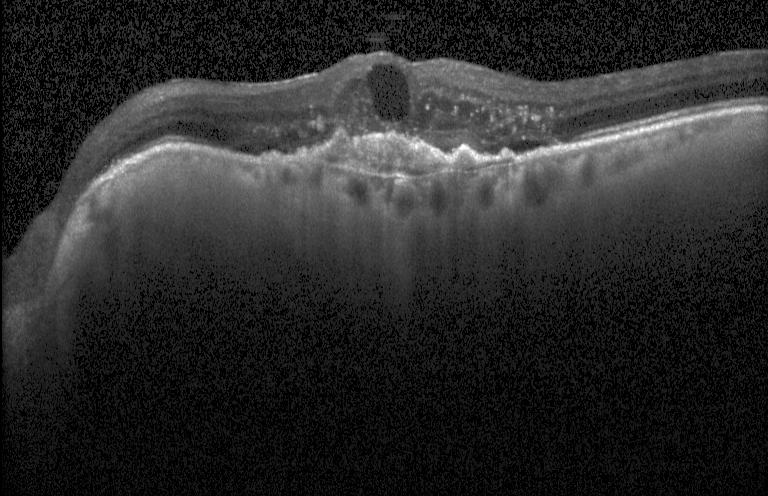 Macular OCT: a choroidal neovascular membrane.